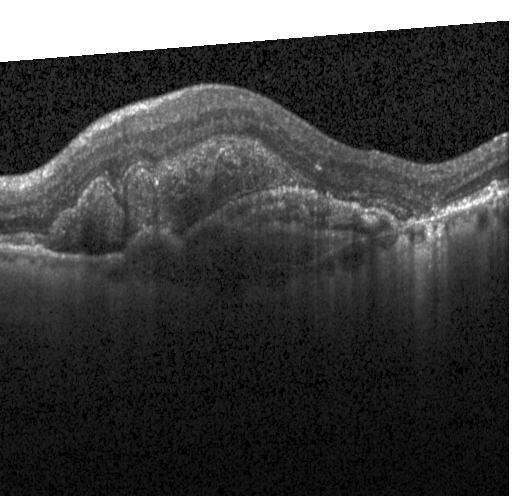 Finding: CNV.